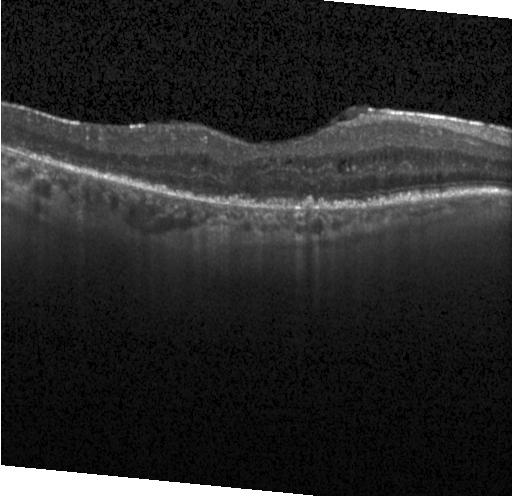 Macular scan; optical coherence tomography scan
Impression: neither choroidal neovascularization, diabetic macular edema, nor drusen.